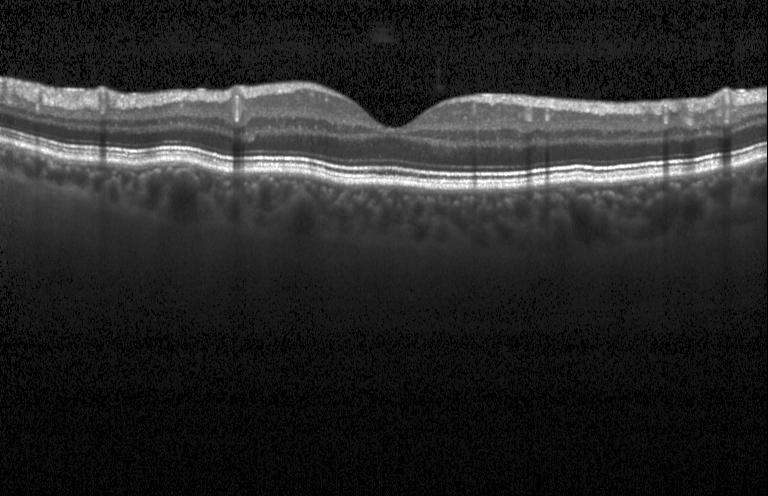

Retinal OCT cross-section.
Finding: neither choroidal neovascularization, diabetic macular edema, nor drusen.